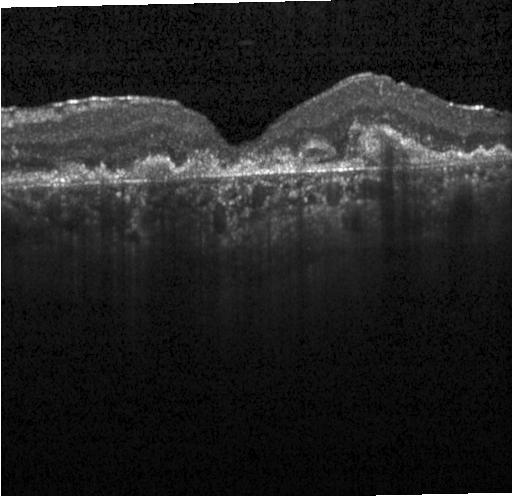

OCT line scan, spectral-domain OCT — Assessment: a choroidal neovascular membrane.